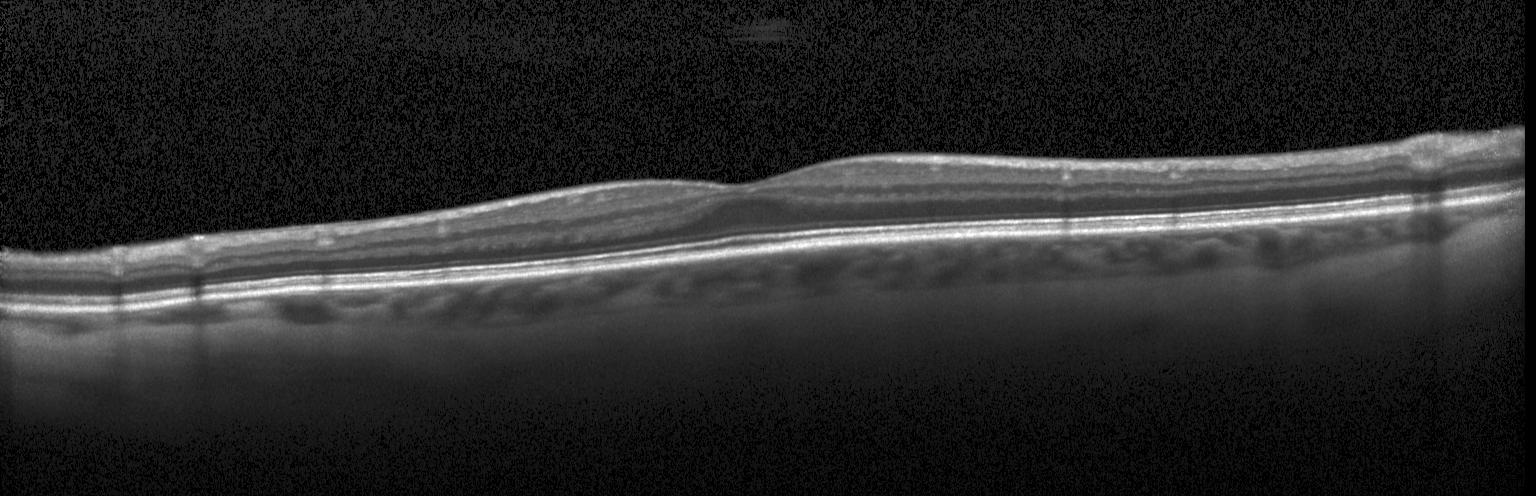

Impression: no choroidal neovascularization, diabetic macular edema, or drusen.